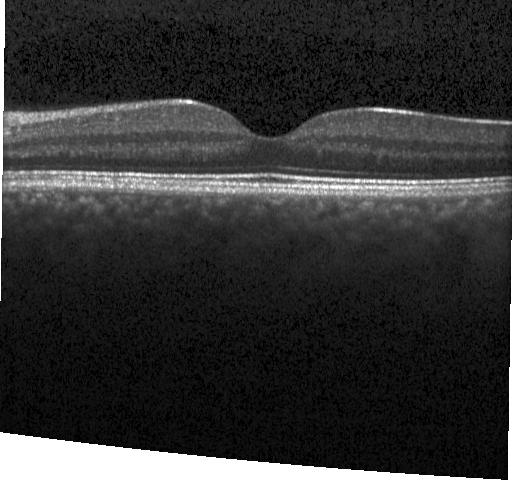
Retinal OCT B-scan — Impression: neither choroidal neovascularization, diabetic macular edema, nor drusen.